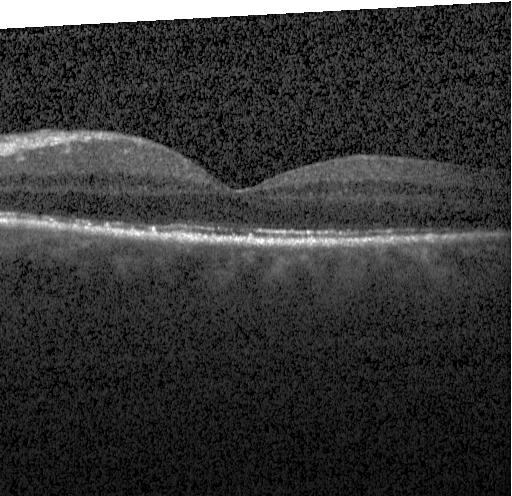 OCT B-scan, spectral-domain OCT, centered on the fovea — No choroidal neovascularization, no diabetic macular edema, and no drusen.